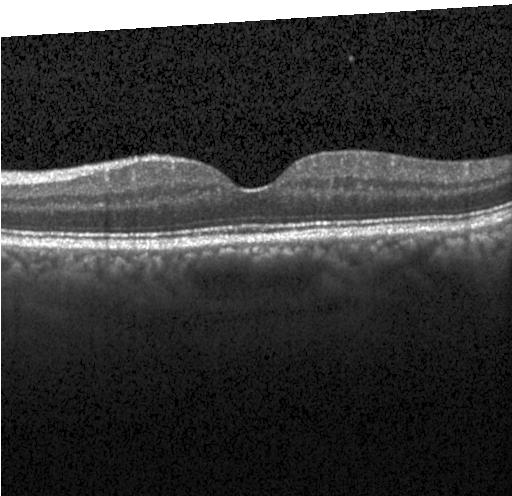
Impression: no evidence of choroidal neovascularization, diabetic macular edema, or drusen.